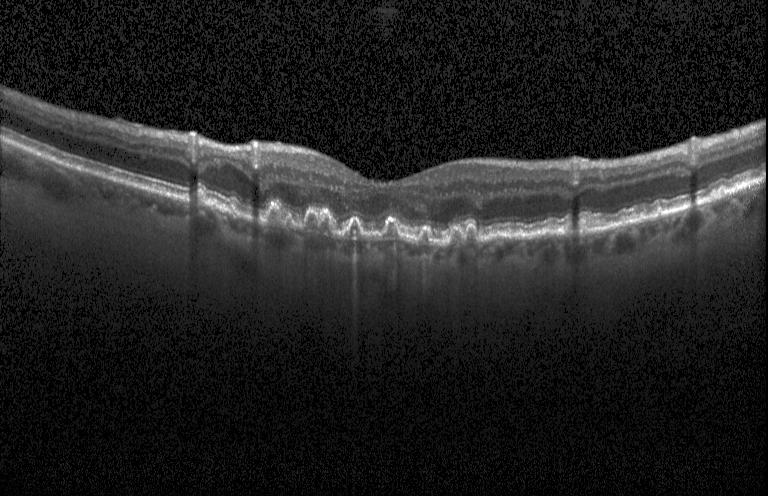 SD-OCT; horizontal scan through the fovea; optical coherence tomography B-scan; Heidelberg Spectralis OCT system. Finding: sub-RPE drusenoid deposits.